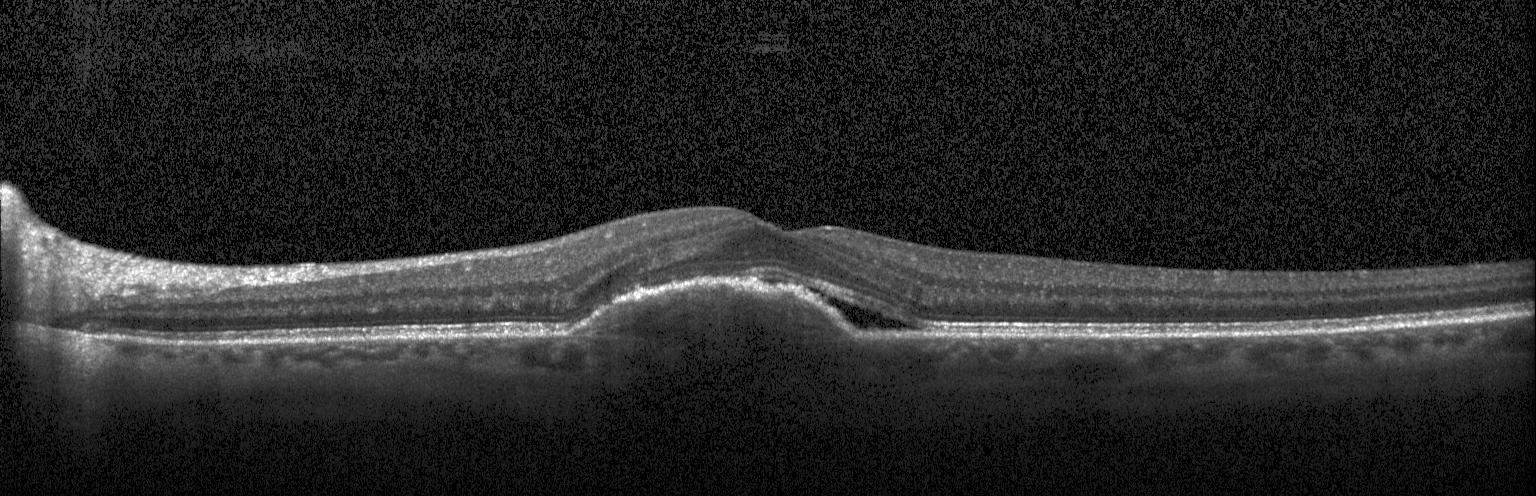 Macular OCT: a choroidal neovascular membrane.